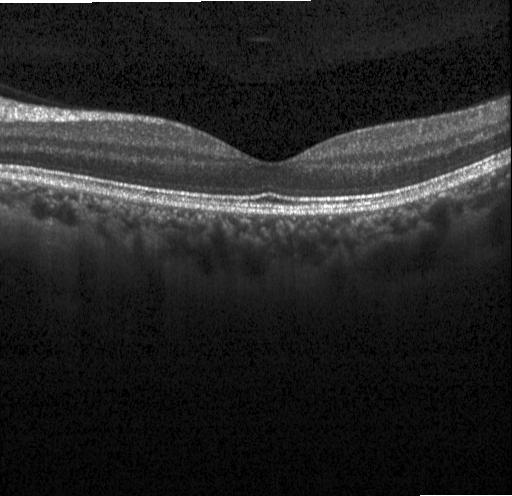

Retinal OCT cross-section — Diagnosis: no choroidal neovascularization, diabetic macular edema, or drusen.